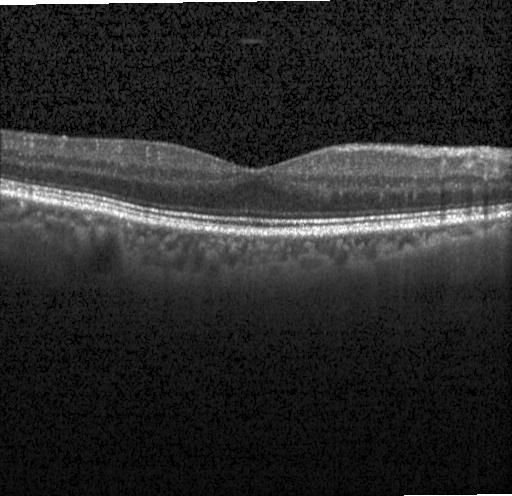 Assessment: neither CNV, DME, nor drusen.